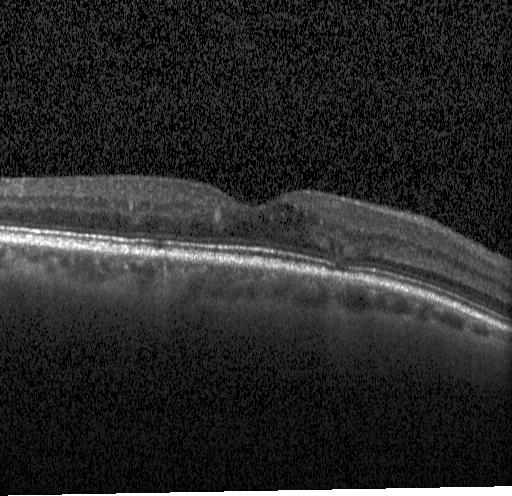

Macular OCT: diabetic macular edema (DME).